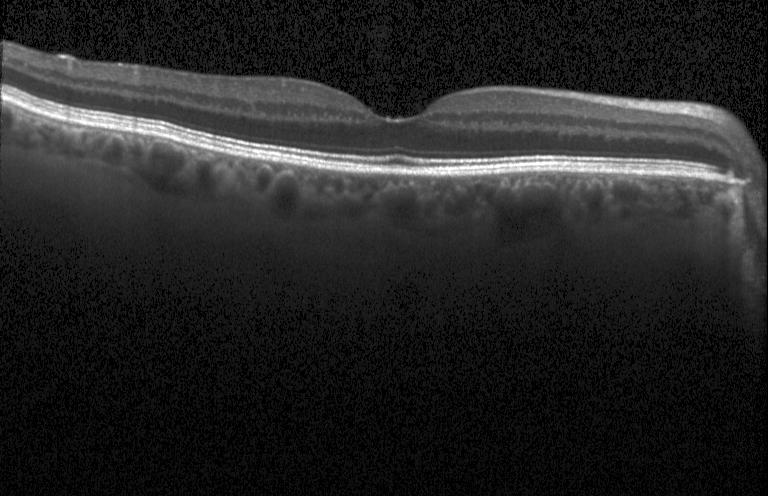
Spectral-domain OCT. Centered on the fovea. Optical coherence tomography B-scan. Heidelberg Spectralis OCT system — Assessment: no evidence of choroidal neovascularization, diabetic macular edema, or drusen.